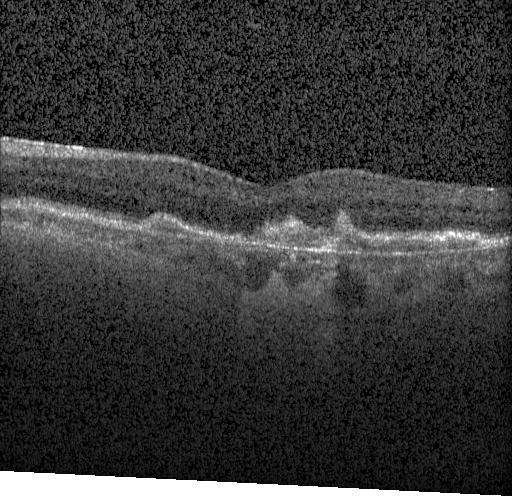
Instrument: Heidelberg Spectralis · optical coherence tomography B-scan · SD-OCT — Diagnosis: choroidal neovascularization (CNV).